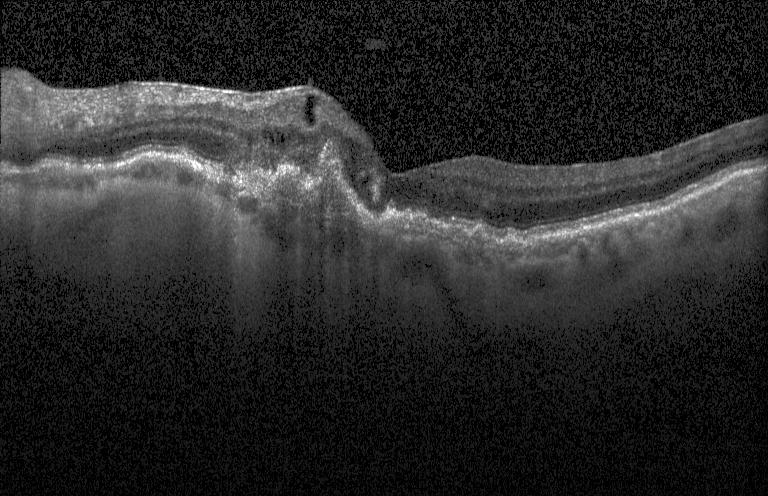
Spectral-domain OCT, Heidelberg Spectralis OCT system, fovea-centered, optical coherence tomography B-scan
Finding: choroidal neovascularization (CNV).